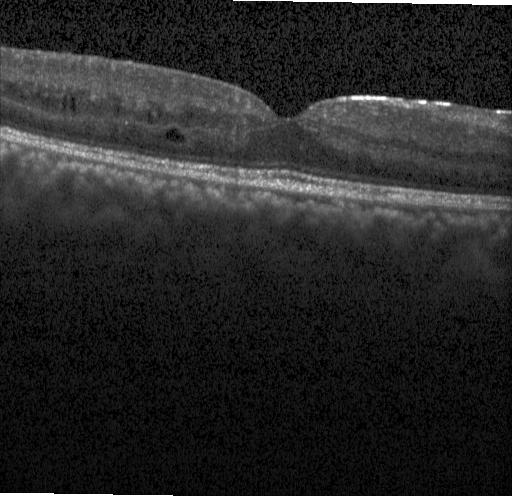
Retinal OCT cross-section. Finding: DME.